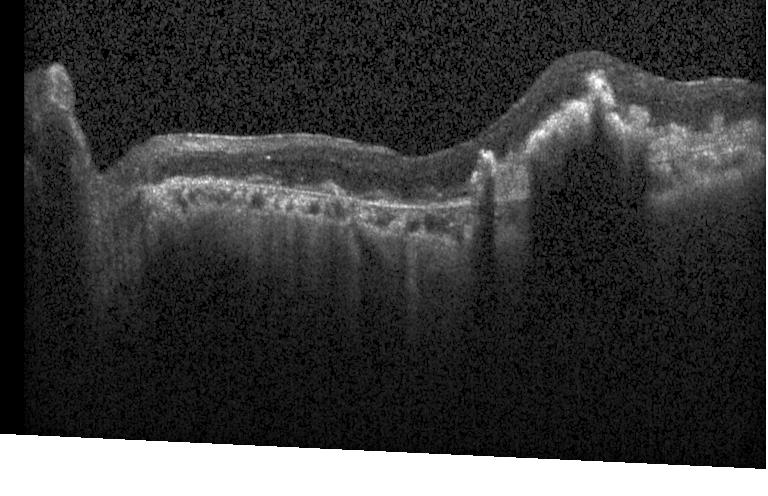

Assessment: choroidal neovascularization (CNV).